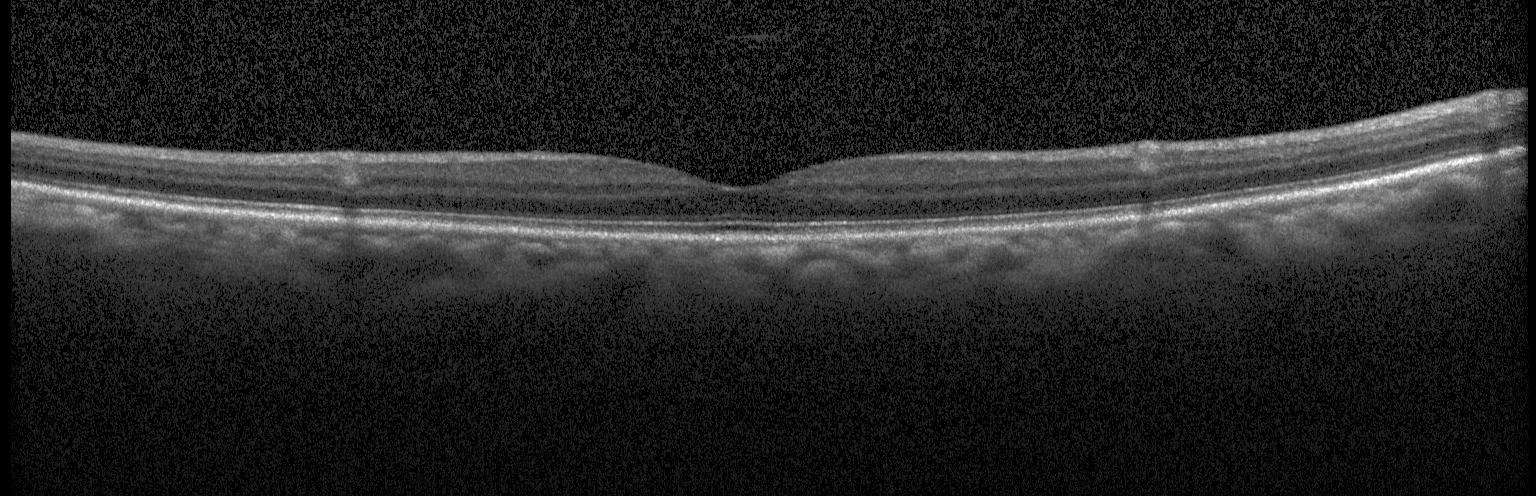
Instrument: Heidelberg Spectralis · fovea-centered · retinal OCT B-scan · SD-OCT
Diagnosis: neither choroidal neovascularization, diabetic macular edema, nor drusen.